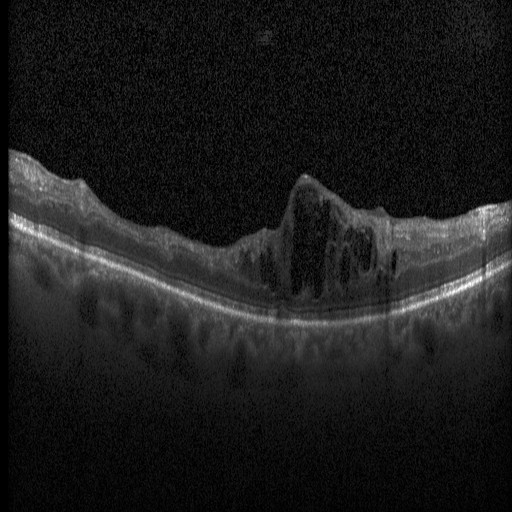

Spectral-domain OCT. Instrument: Heidelberg Spectralis. OCT line scan. Fovea-centered
Assessment: diabetic macular edema (DME).